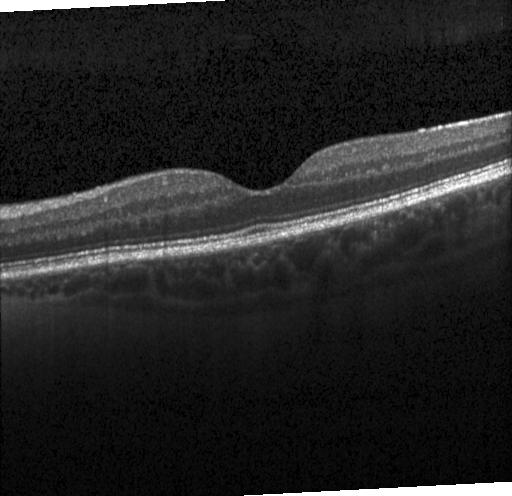 Spectral-domain OCT B-scan: no choroidal neovascularization, no diabetic macular edema, and no drusen.